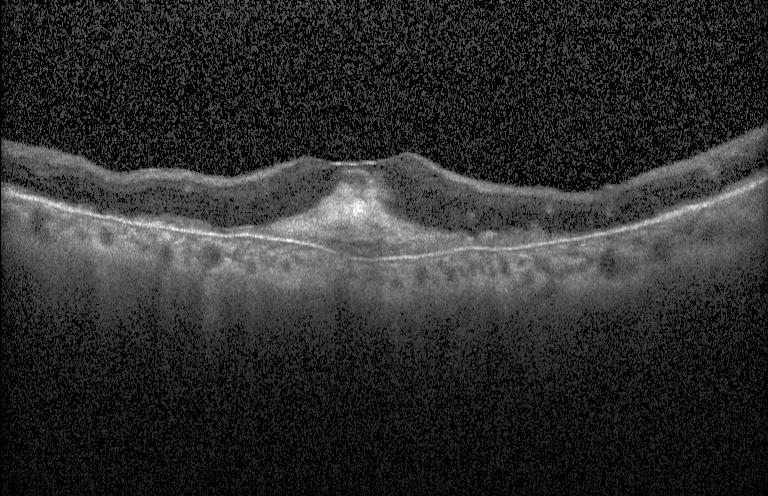 OCT B-scan · instrument: Heidelberg Spectralis — Dx: choroidal neovascularization (CNV).